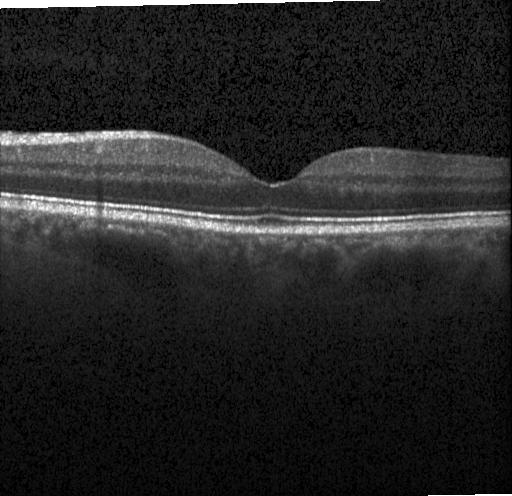

OCT line scan. Dx: neither choroidal neovascularization, diabetic macular edema, nor drusen.